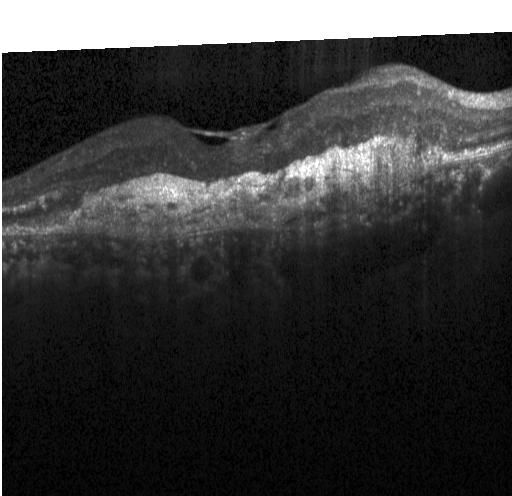

Horizontal scan through the fovea · Heidelberg Spectralis OCT system · spectral-domain optical coherence tomography · OCT B-scan
Diagnosis: a choroidal neovascular membrane.